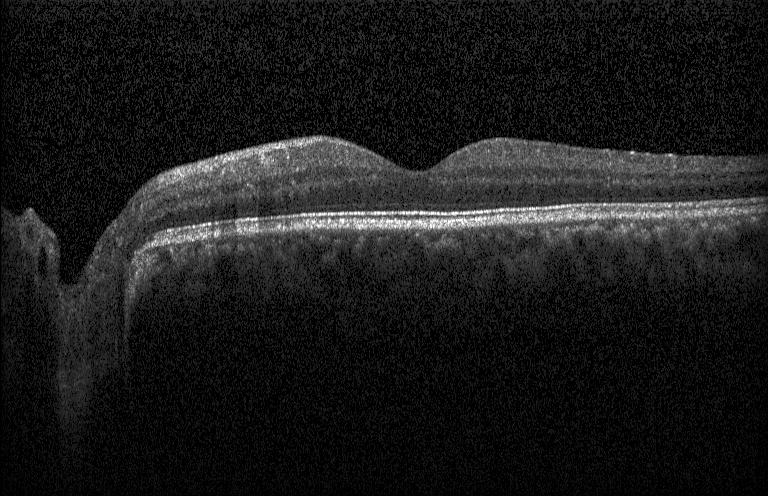

OCT B-scan showing no choroidal neovascularization, diabetic macular edema, or drusen.